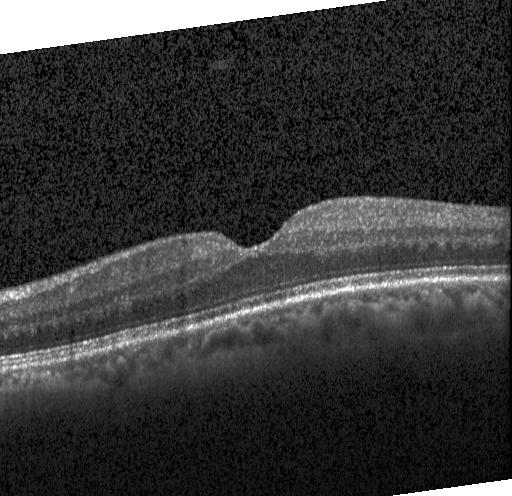
Finding: no evidence of choroidal neovascularization, diabetic macular edema, or drusen.